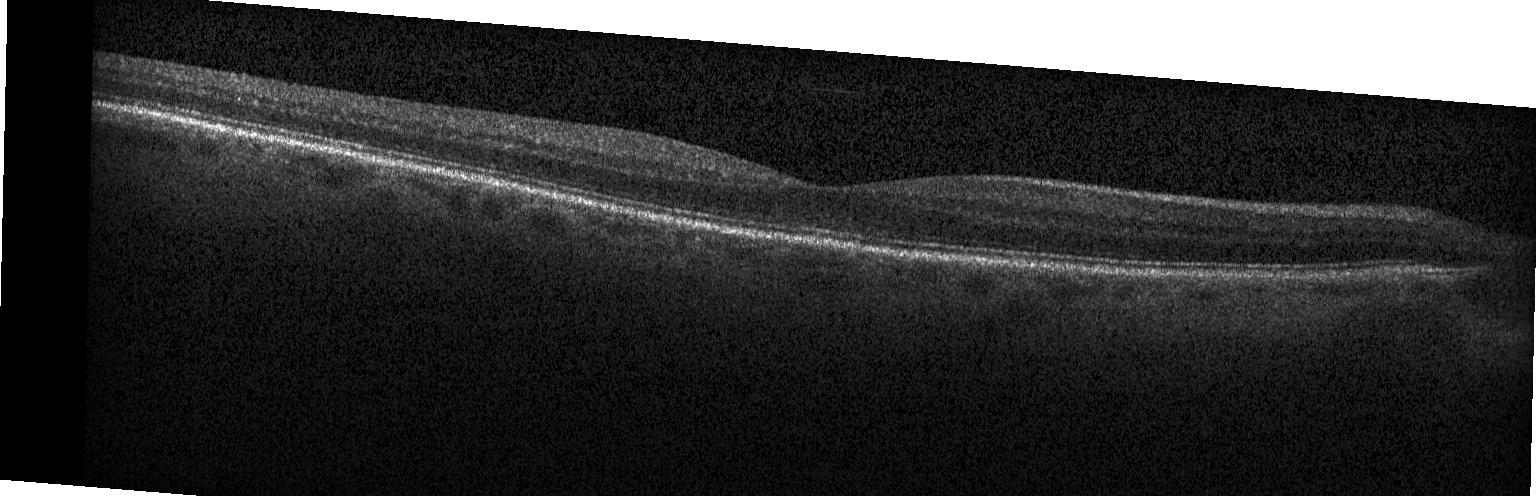 Finding: neither choroidal neovascularization, diabetic macular edema, nor drusen.